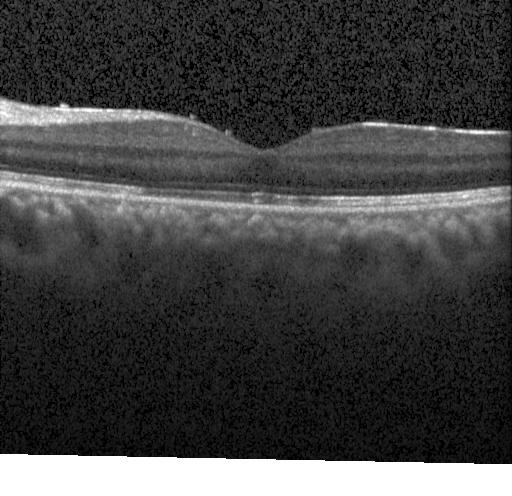

OCT B-scan; Heidelberg Spectralis OCT system. Macular OCT: no CNV, DME, or drusen.